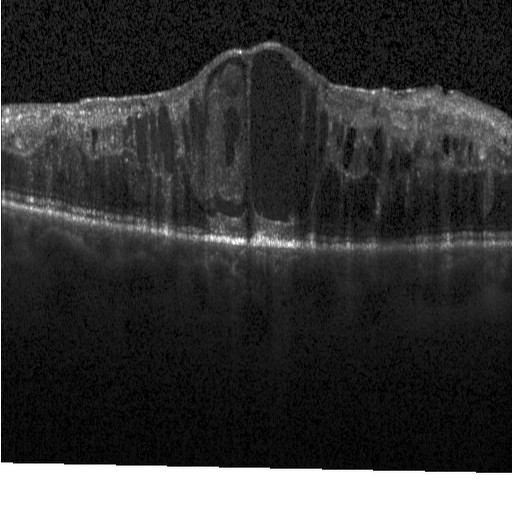

Macular scan. SD-OCT. Retinal OCT B-scan
The scan shows diabetic macular edema.